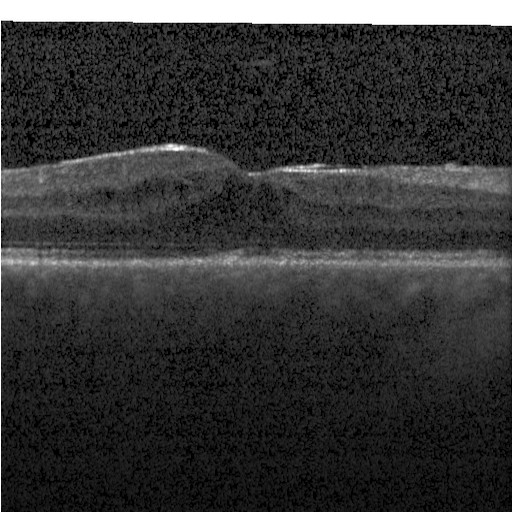

Optical coherence tomography B-scan
Finding: diabetic macular edema (DME).